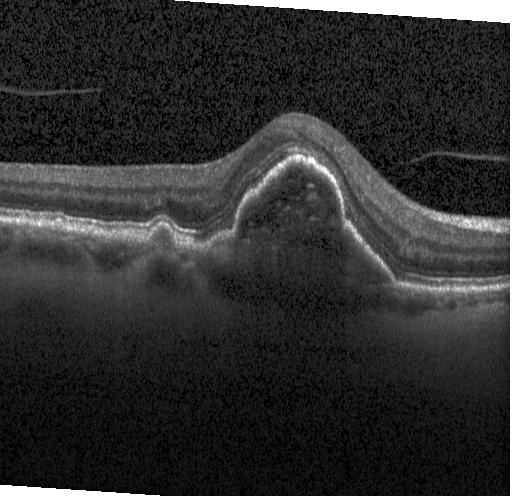
Macular OCT demonstrating CNV.